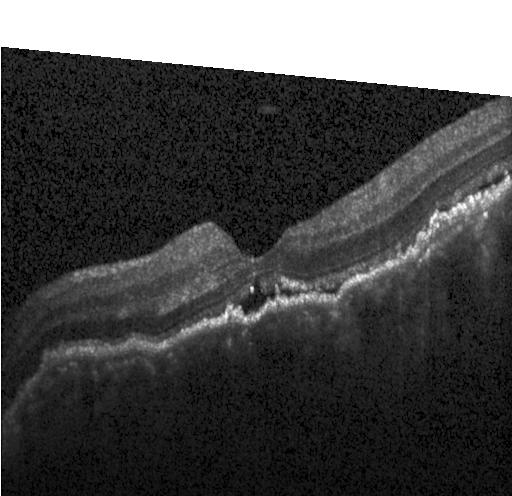 Impression: a choroidal neovascular membrane.